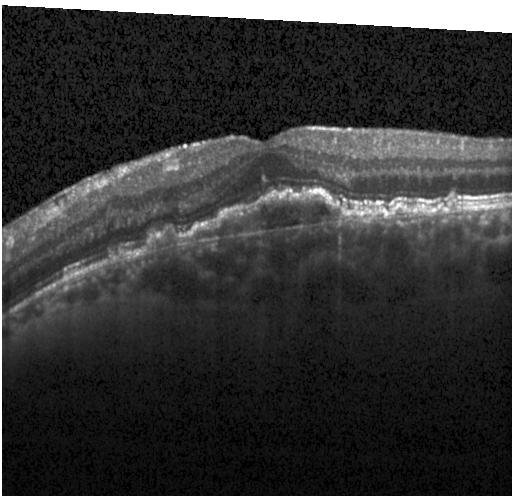 Assessment: a choroidal neovascular membrane.